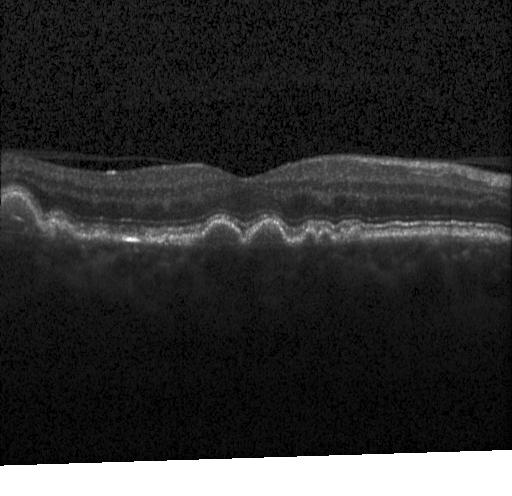
Spectral-domain optical coherence tomography; retinal OCT cross-section; horizontal scan through the fovea; instrument: Heidelberg Spectralis
This B-scan demonstrates sub-RPE drusenoid deposits.